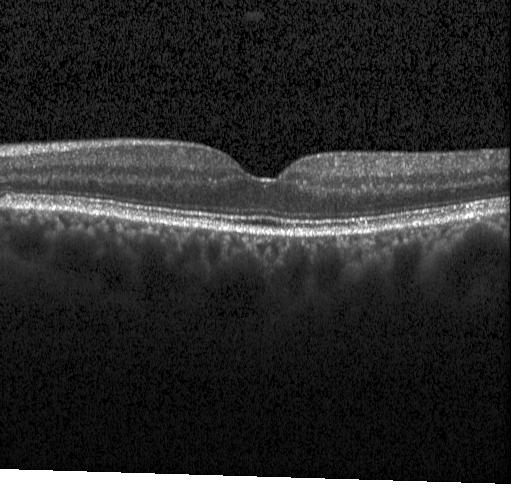

OCT line scan. Spectral-domain OCT.
Diagnosis: no CNV, DME, or drusen.